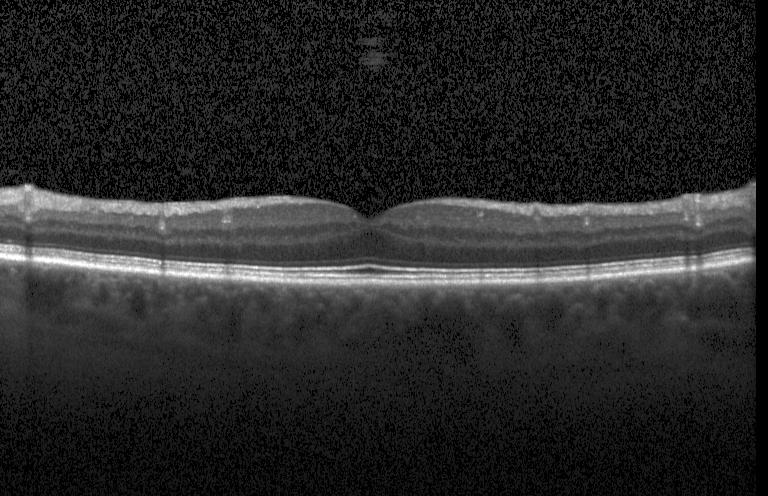
Optical coherence tomography scan, Heidelberg Spectralis, centered on the fovea. Finding: neither CNV, DME, nor drusen.